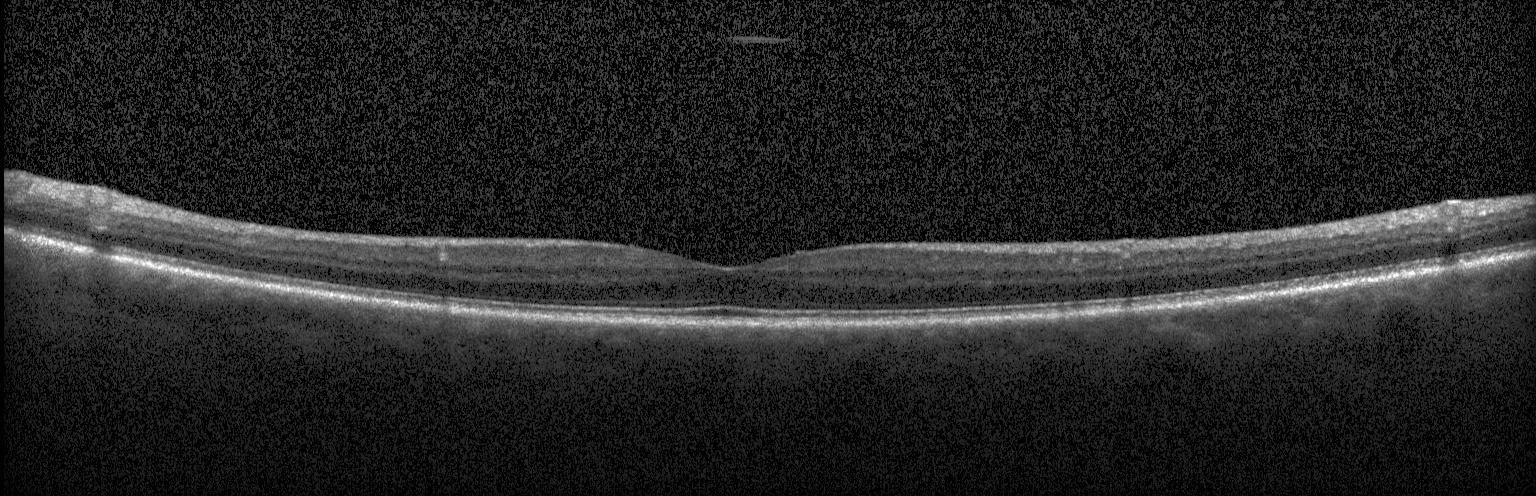 Optical coherence tomography B-scan. Through the macula. Heidelberg Spectralis. SD-OCT
Diagnosis: no choroidal neovascularization, no diabetic macular edema, and no drusen.